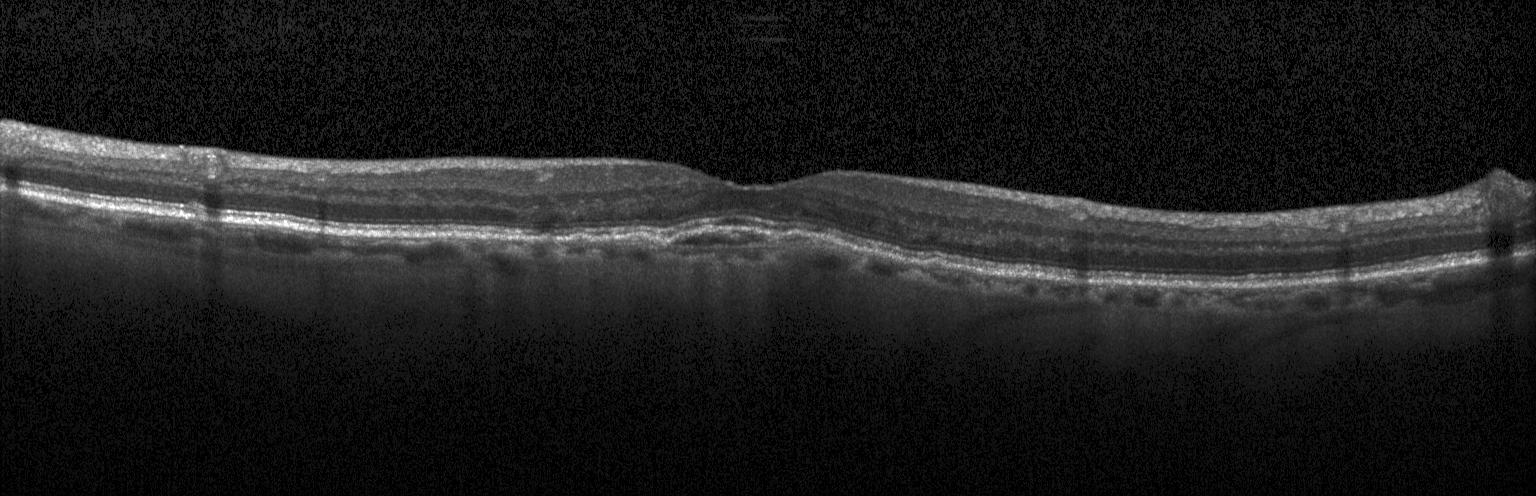
Macular OCT: CNV.